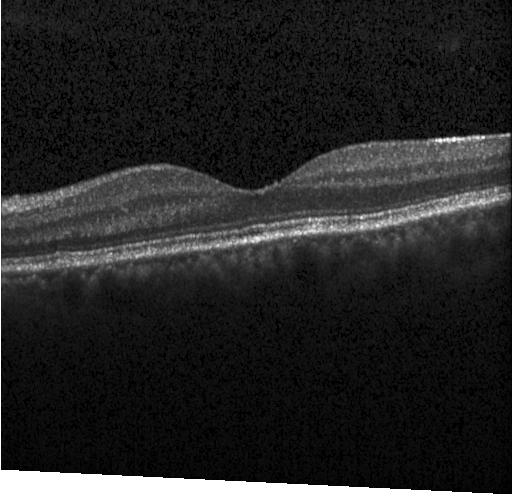

Retinal OCT B-scan. Finding: no evidence of CNV, DME, or drusen.